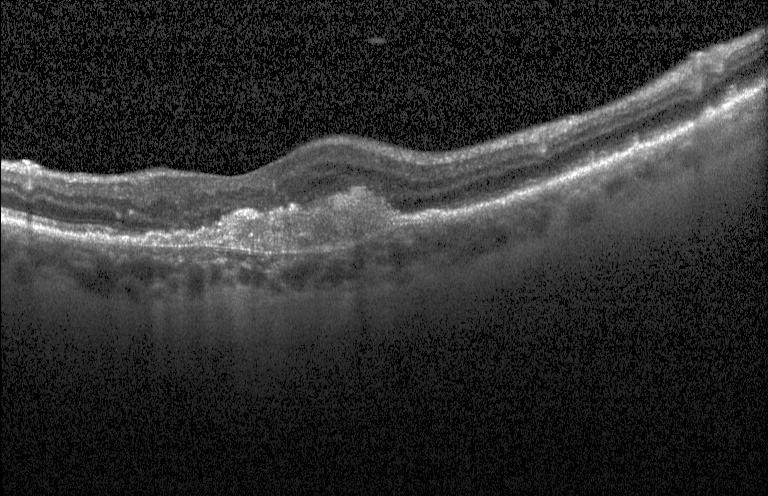
Diagnosis: choroidal neovascularization.